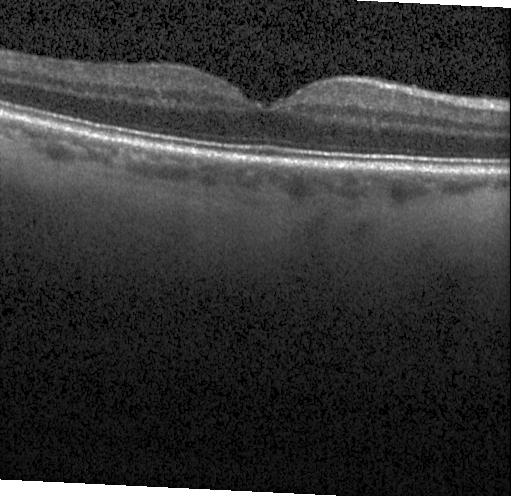
Retinal OCT cross-section — Dx: no choroidal neovascularization, diabetic macular edema, or drusen.